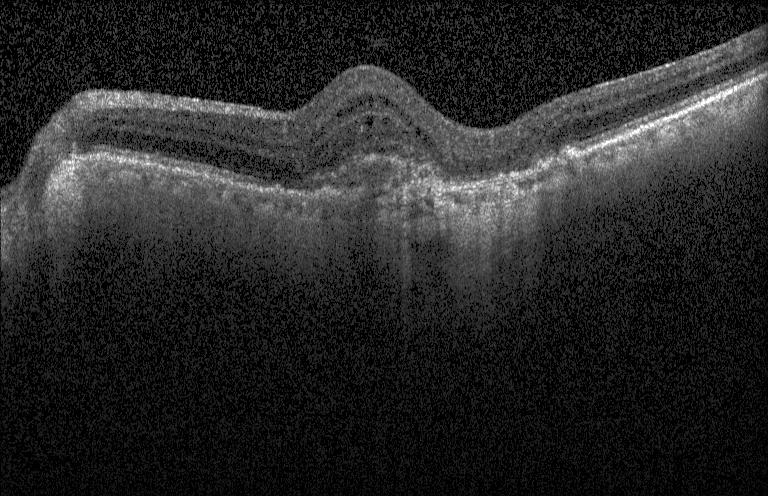
Retinal OCT cross-section · macular scan · Heidelberg Spectralis OCT system.
Finding: CNV.